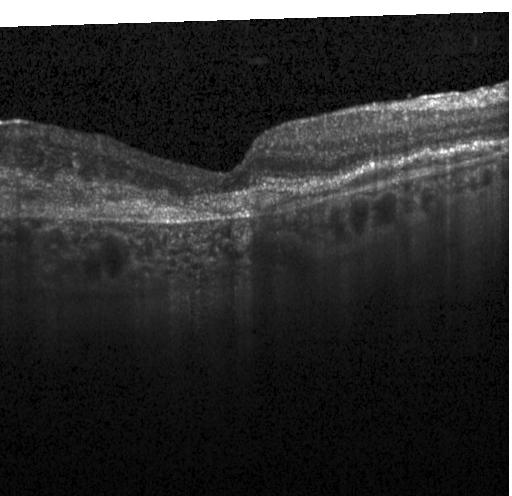

Spectral-domain OCT, retinal OCT B-scan — This B-scan demonstrates choroidal neovascularization (CNV).